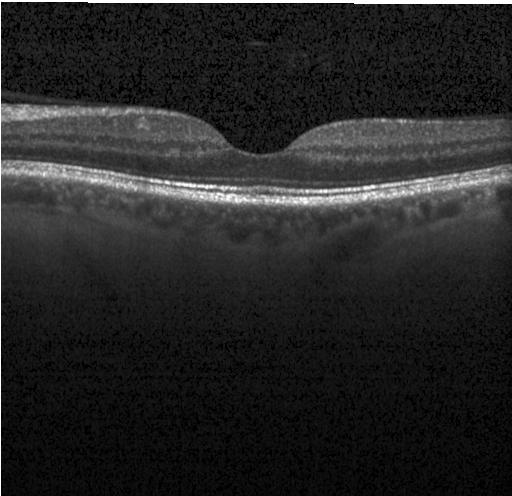 Finding: no evidence of choroidal neovascularization, diabetic macular edema, or drusen.